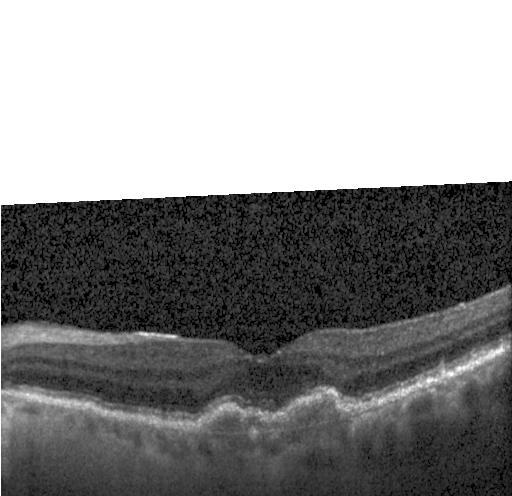 Retinal OCT B-scan; Heidelberg Spectralis OCT system; through the macula. Diagnosis: choroidal neovascularization.